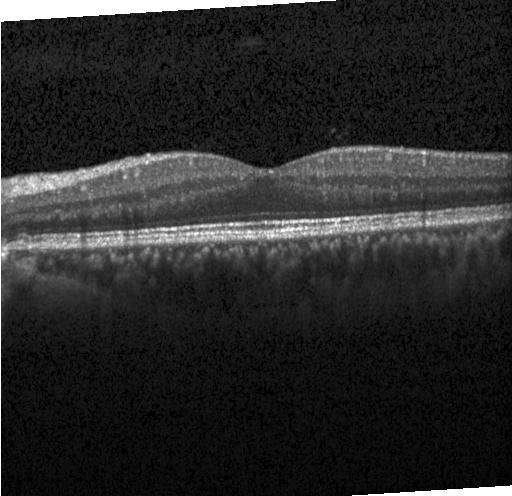 Macular OCT: no choroidal neovascularization, no diabetic macular edema, and no drusen.